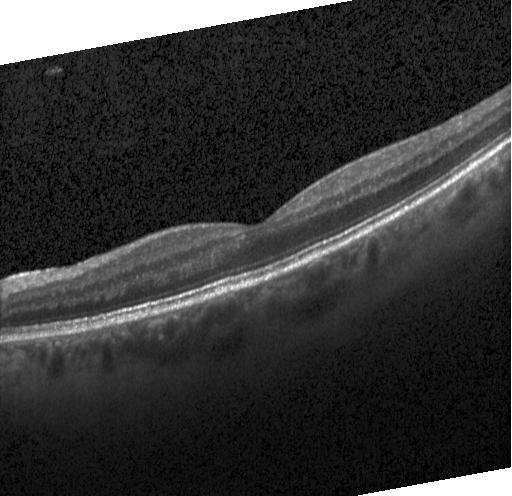

Optical coherence tomography B-scan
The scan shows no choroidal neovascularization, no diabetic macular edema, and no drusen.